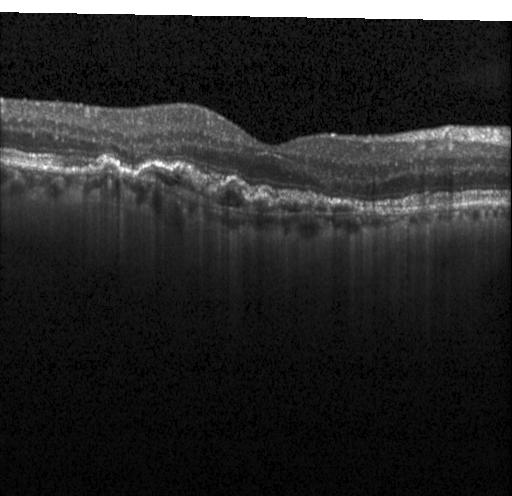 Spectral-domain optical coherence tomography. Through the macula. OCT B-scan. Diagnosis: choroidal neovascularization (CNV).